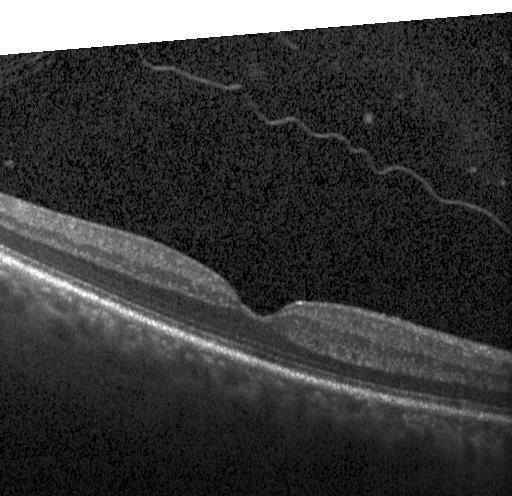
Optical coherence tomography scan
Finding: neither choroidal neovascularization, diabetic macular edema, nor drusen.